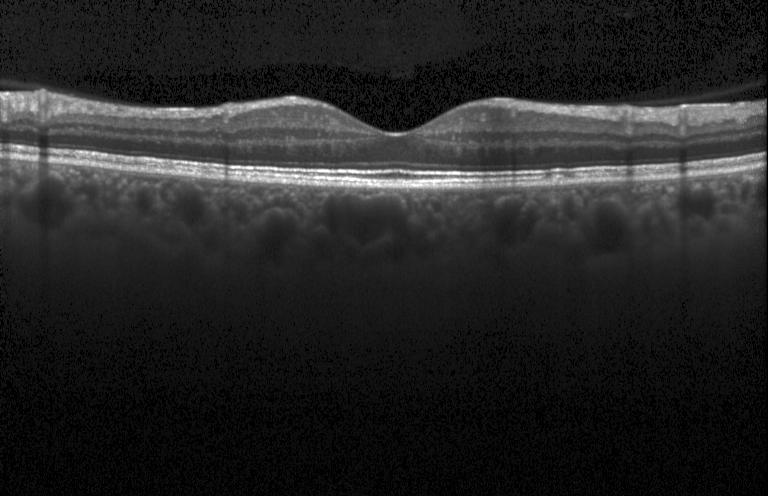 Dx: no CNV, DME, or drusen.